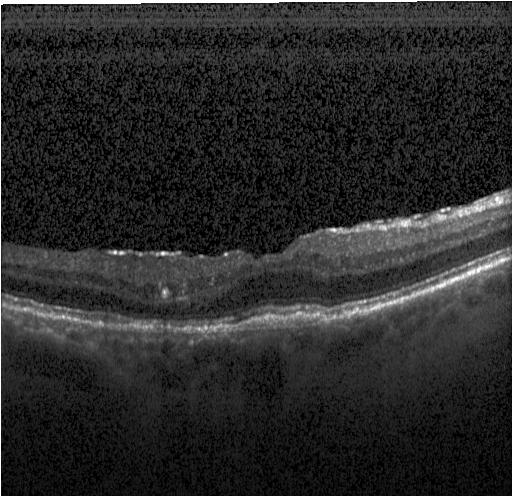
Optical coherence tomography B-scan; SD-OCT.
Assessment: a choroidal neovascular membrane.